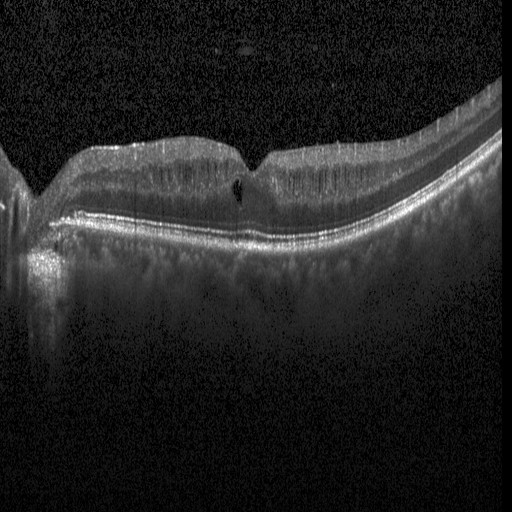

Macular scan, Heidelberg Spectralis, retinal OCT cross-section.
Diagnosis: diabetic macular edema (DME).